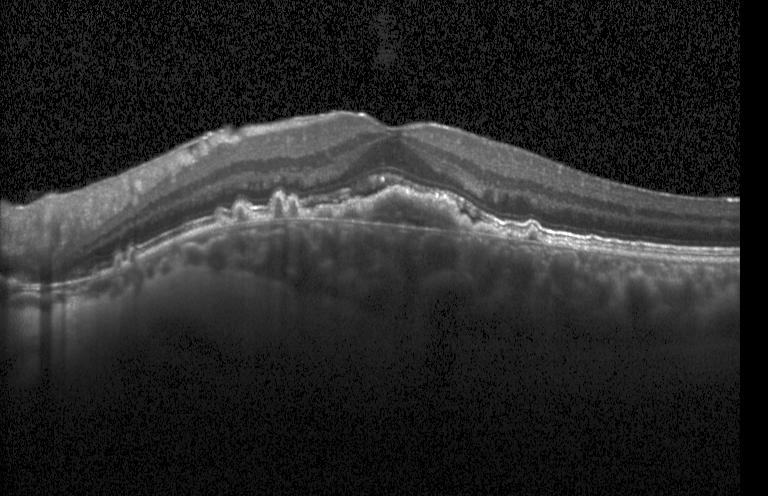 OCT B-scan showing a choroidal neovascular membrane.